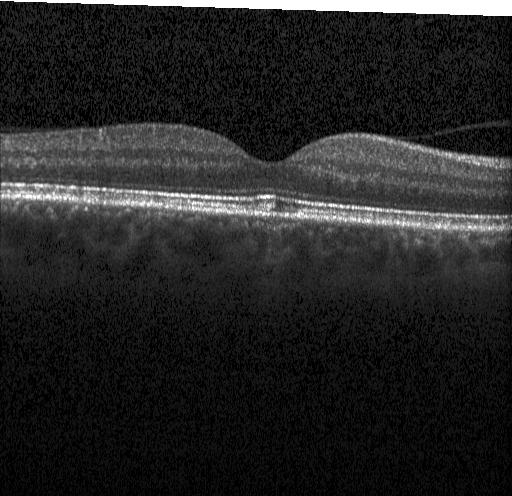

Optical coherence tomography scan; Heidelberg Spectralis OCT system
Assessment: no evidence of choroidal neovascularization, diabetic macular edema, or drusen.